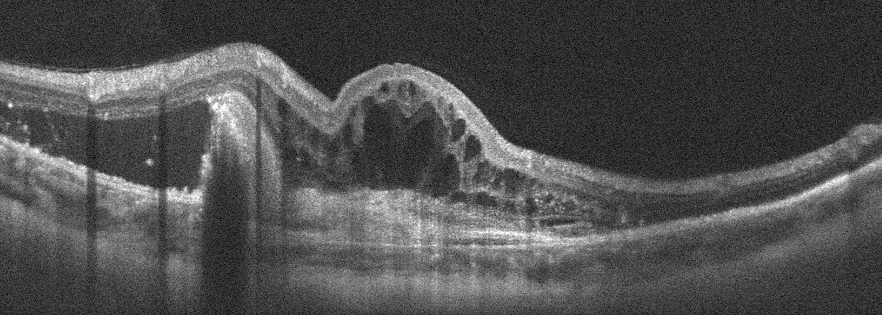 Optical coherence tomography B-scan; right eye; acquired on an Optovue Avanti RTVue XR; macular scan
Diagnosis: age-related macular degeneration (AMD).